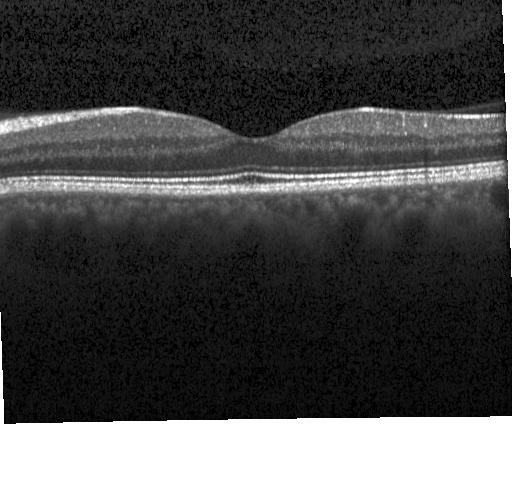

Retinal OCT cross-section — Finding: no choroidal neovascularization, diabetic macular edema, or drusen.